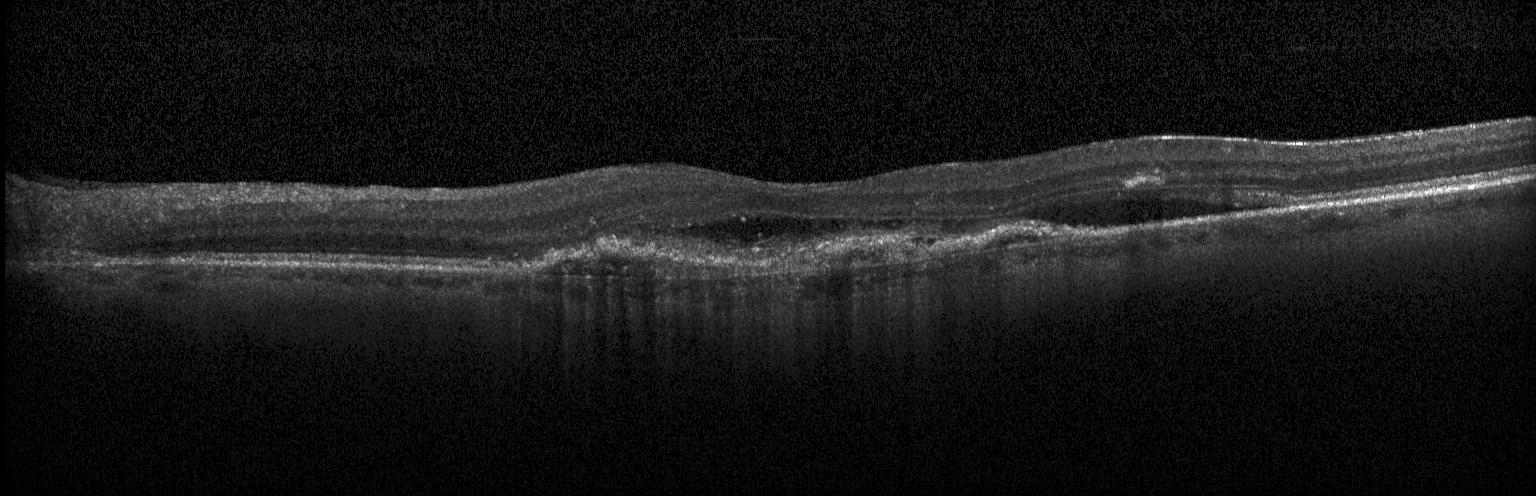

Through the macula. Retinal OCT cross-section.
Macular OCT: choroidal neovascularization.